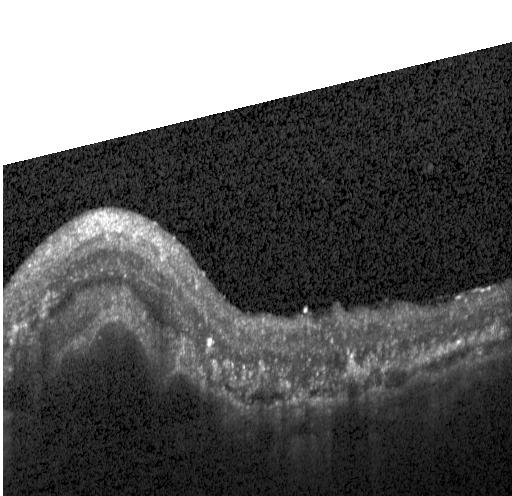

Dx: a choroidal neovascular membrane.